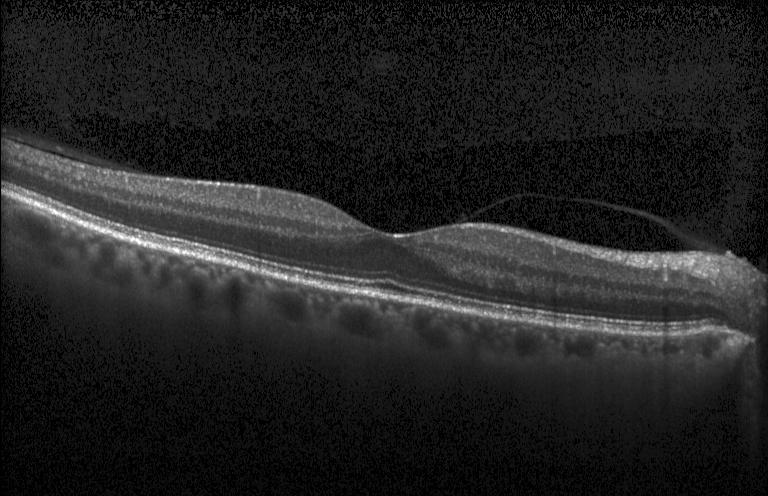
Fovea-centered · acquired on a Heidelberg Spectralis · retinal OCT B-scan · spectral-domain optical coherence tomography — This B-scan demonstrates no choroidal neovascularization, diabetic macular edema, or drusen.